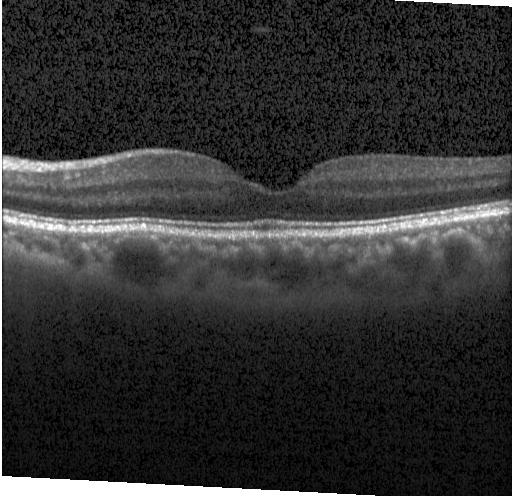

OCT B-scan
No choroidal neovascularization, diabetic macular edema, or drusen.